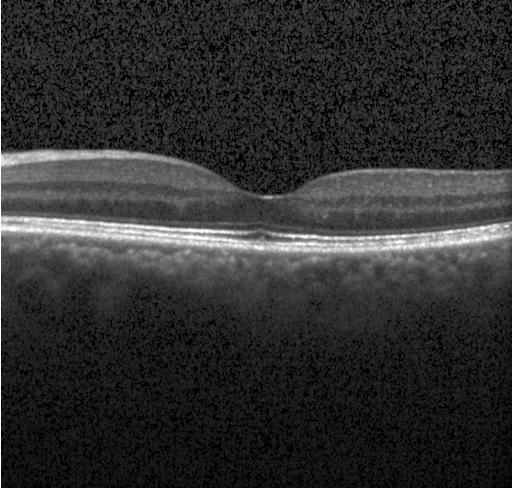

Finding: no choroidal neovascularization, diabetic macular edema, or drusen.